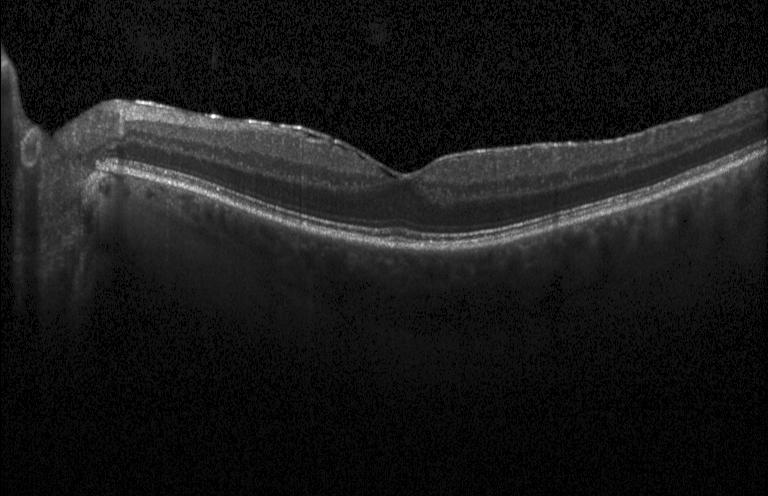 OCT scan showing no evidence of CNV, DME, or drusen.